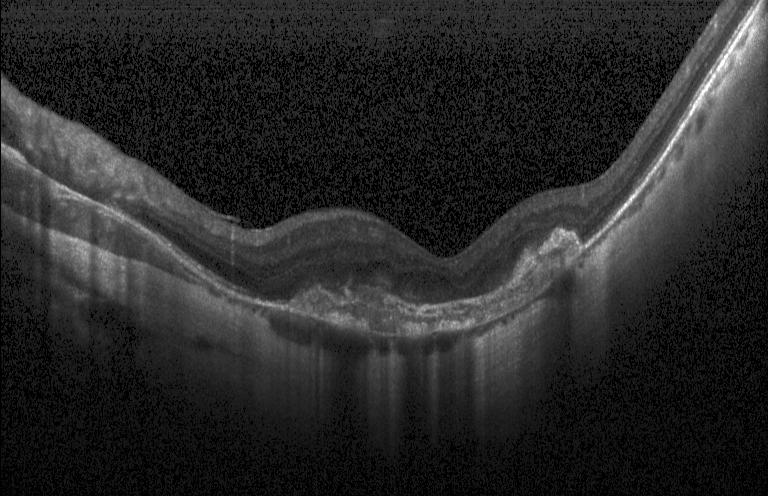 Macular scan, OCT B-scan
Diagnosis: a choroidal neovascular membrane.